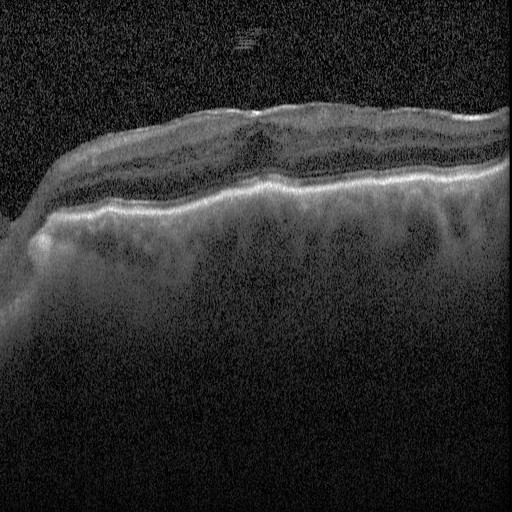
Retinal OCT cross-section showing DME.